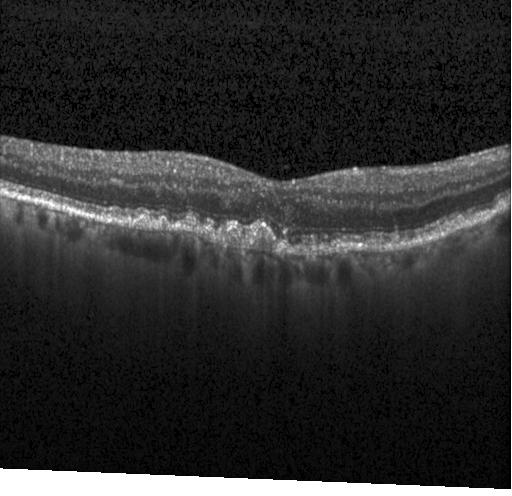
Optical coherence tomography scan. Through the macula
Impression: drusen.